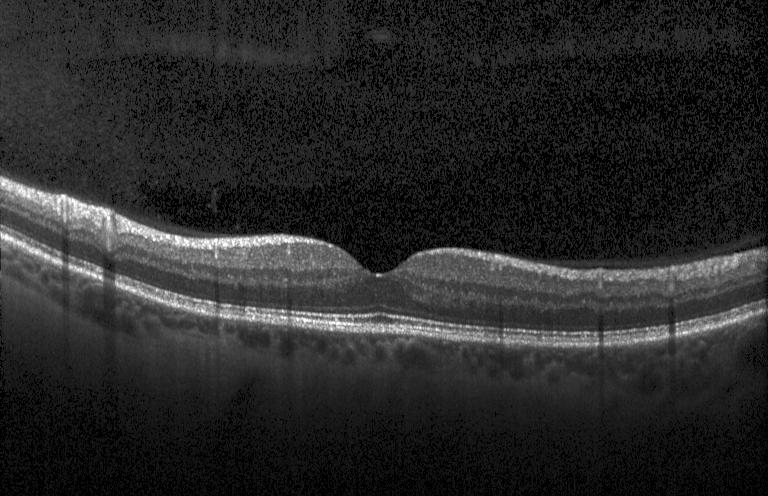

Finding: no evidence of CNV, DME, or drusen.